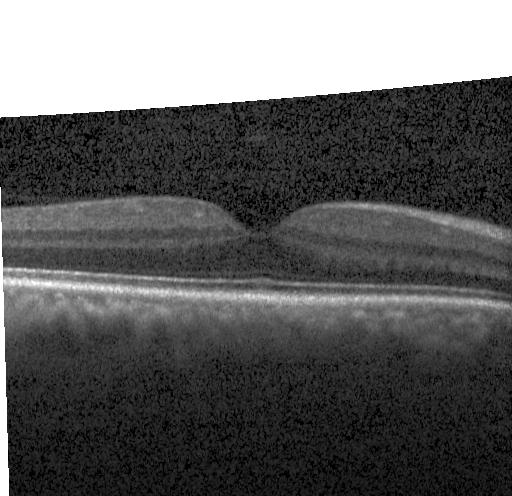
Optical coherence tomography B-scan
The scan shows neither CNV, DME, nor drusen.